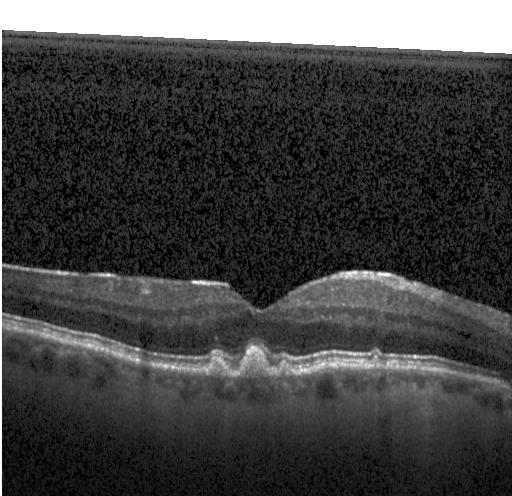
Retinal OCT B-scan, through the macula, SD-OCT, instrument: Heidelberg Spectralis — Dx: drusen.